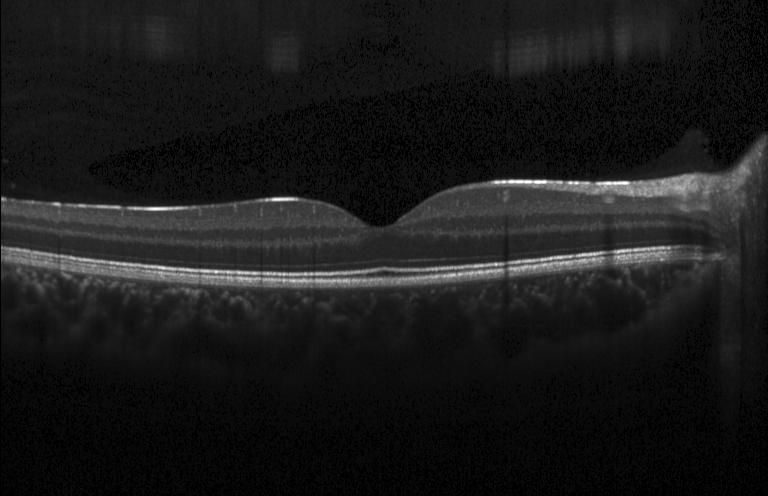

SD-OCT. Heidelberg Spectralis. Optical coherence tomography B-scan.
Diagnosis: neither CNV, DME, nor drusen.